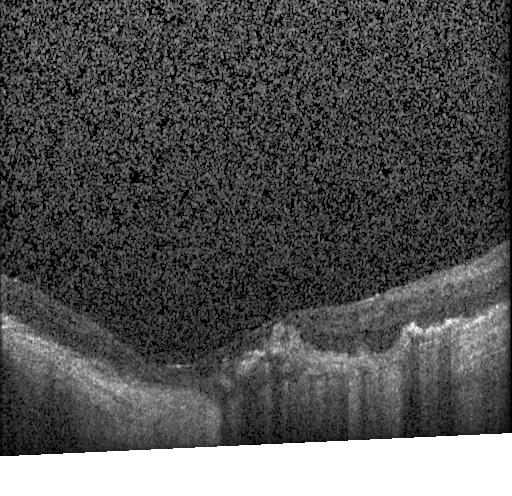
Optical coherence tomography scan. Macular scan.
The scan shows choroidal neovascularization (CNV).